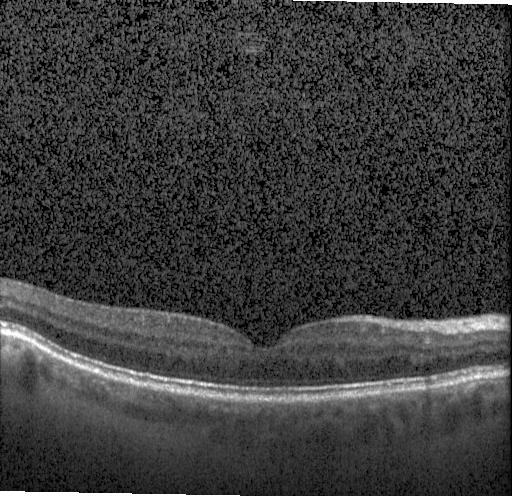

Spectral-domain optical coherence tomography, macular scan, OCT B-scan
Impression: neither choroidal neovascularization, diabetic macular edema, nor drusen.